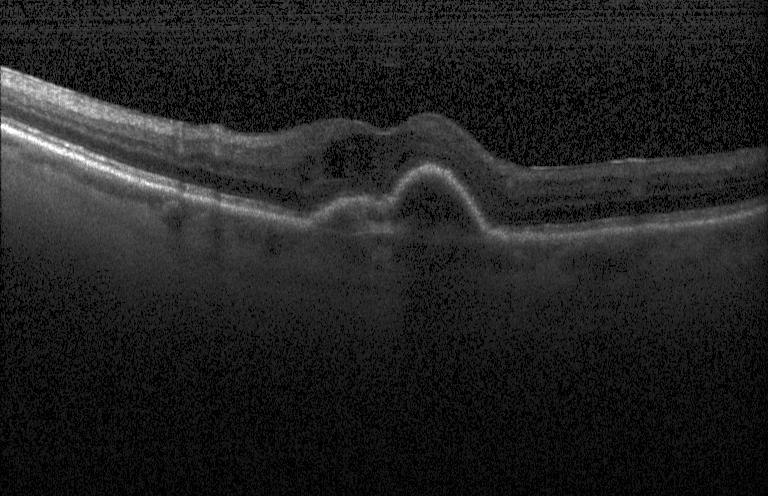 Spectral-domain OCT · OCT B-scan · horizontal scan through the fovea. This B-scan demonstrates a choroidal neovascular membrane.